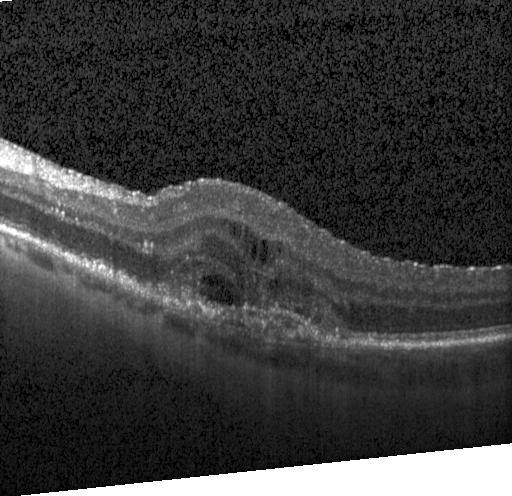
SD-OCT · Heidelberg Spectralis · fovea-centered · OCT B-scan — Impression: CNV.